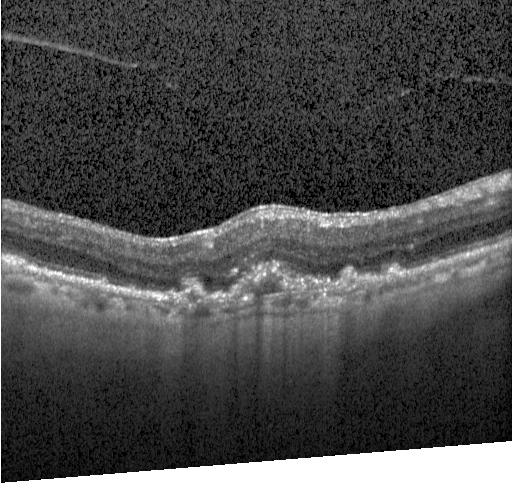 Optical coherence tomography scan
OCT finding: a choroidal neovascular membrane.